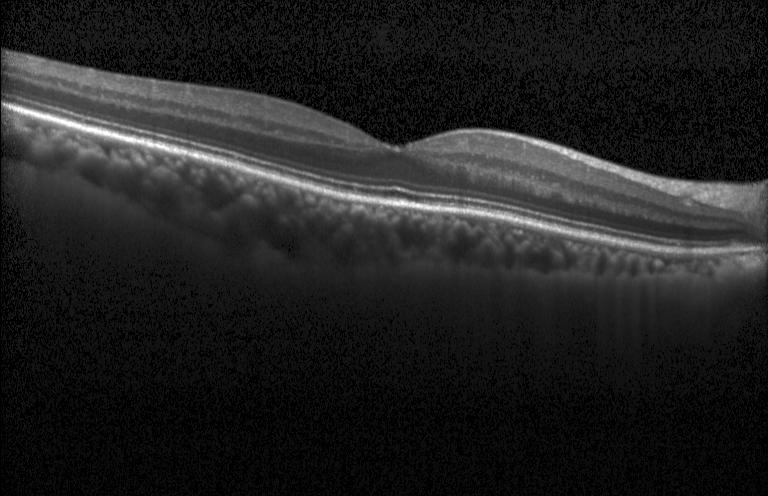
Retinal OCT B-scan · through the macula · Heidelberg Spectralis OCT system
This B-scan demonstrates neither CNV, DME, nor drusen.